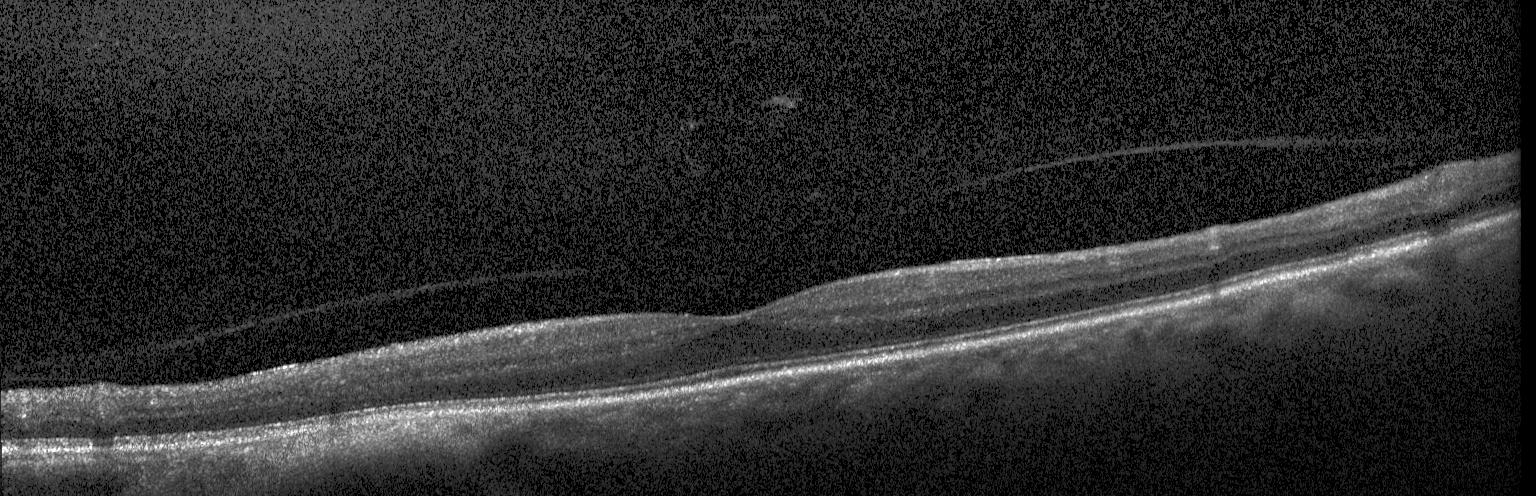
Macular scan · OCT line scan.
OCT finding: neither choroidal neovascularization, diabetic macular edema, nor drusen.